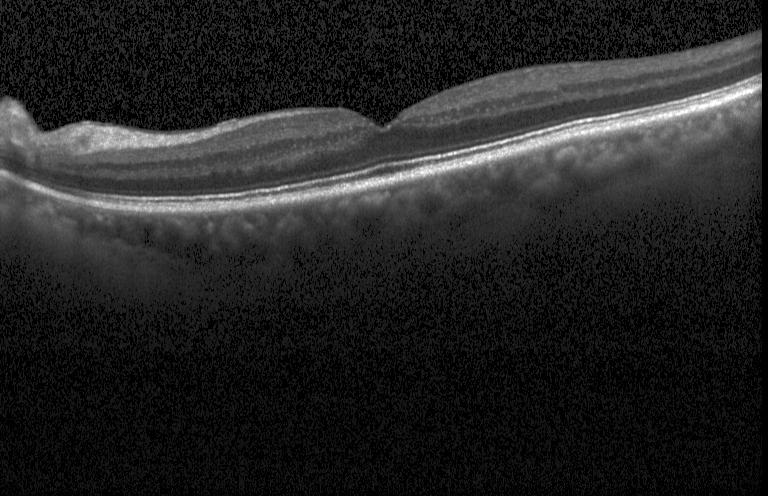
OCT B-scan, instrument: Heidelberg Spectralis, SD-OCT, through the macula.
Assessment: no evidence of CNV, DME, or drusen.